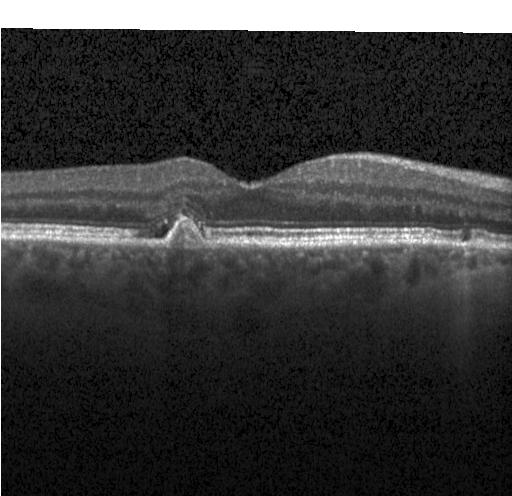

Finding: CNV.